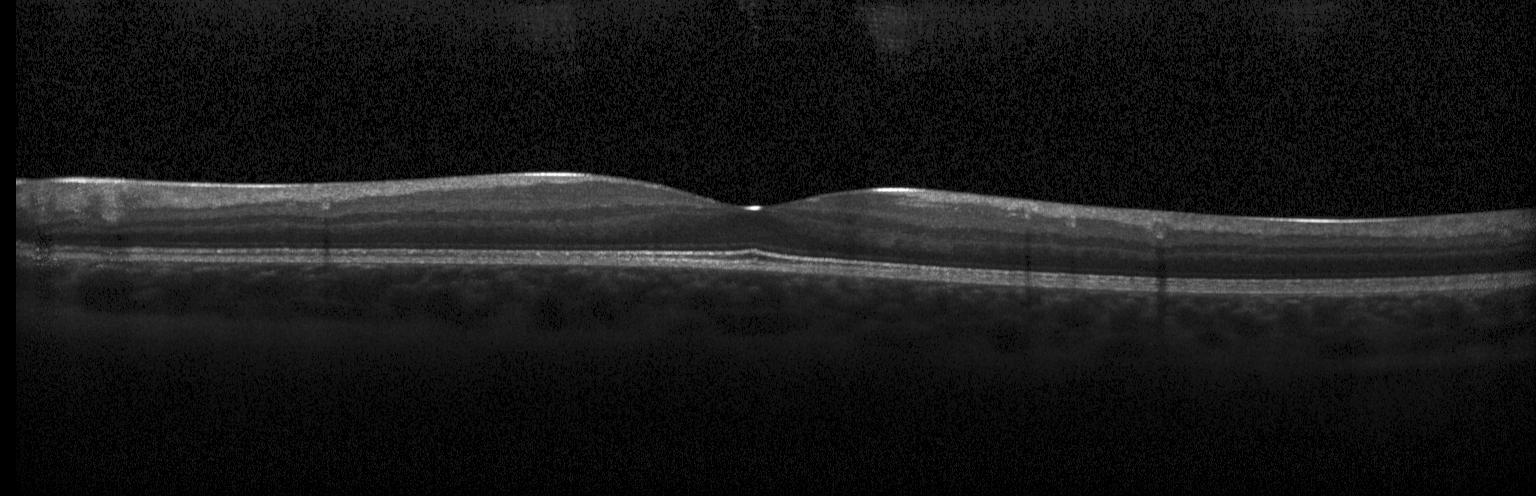

Retinal OCT B-scan. Spectral-domain optical coherence tomography. Instrument: Heidelberg Spectralis.
Impression: no choroidal neovascularization, diabetic macular edema, or drusen.